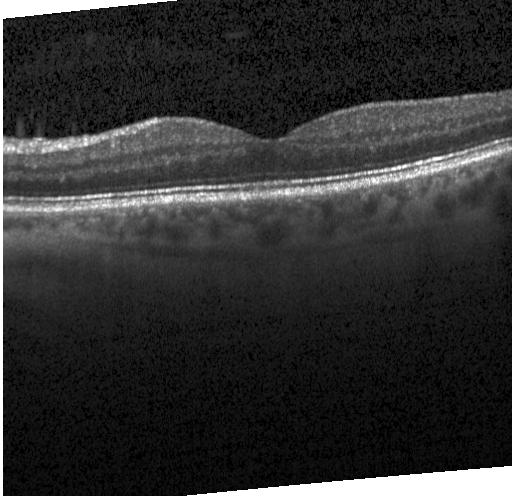
This B-scan demonstrates neither choroidal neovascularization, diabetic macular edema, nor drusen.